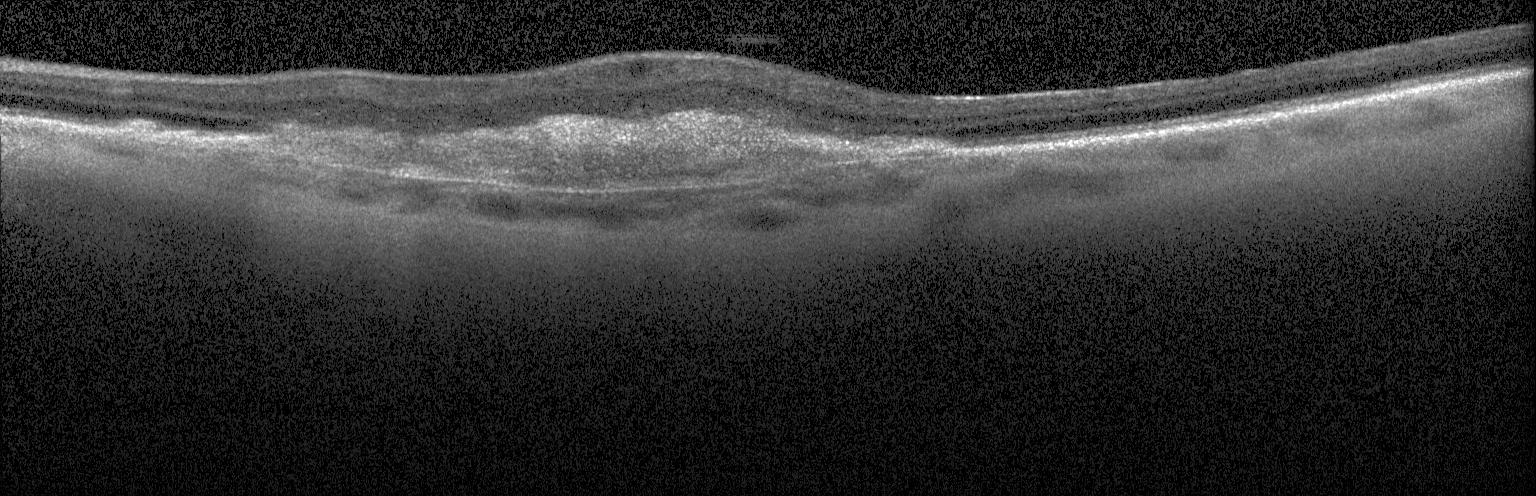 Diagnosis: a choroidal neovascular membrane.